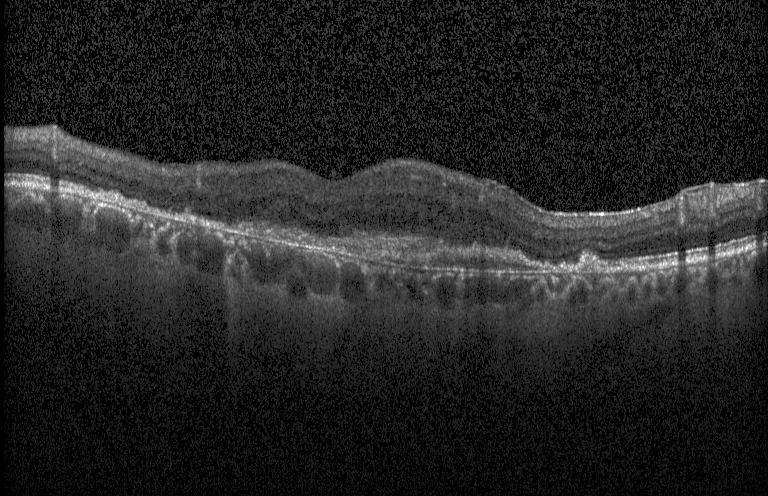
Retinal OCT cross-section.
The scan shows choroidal neovascularization (CNV).